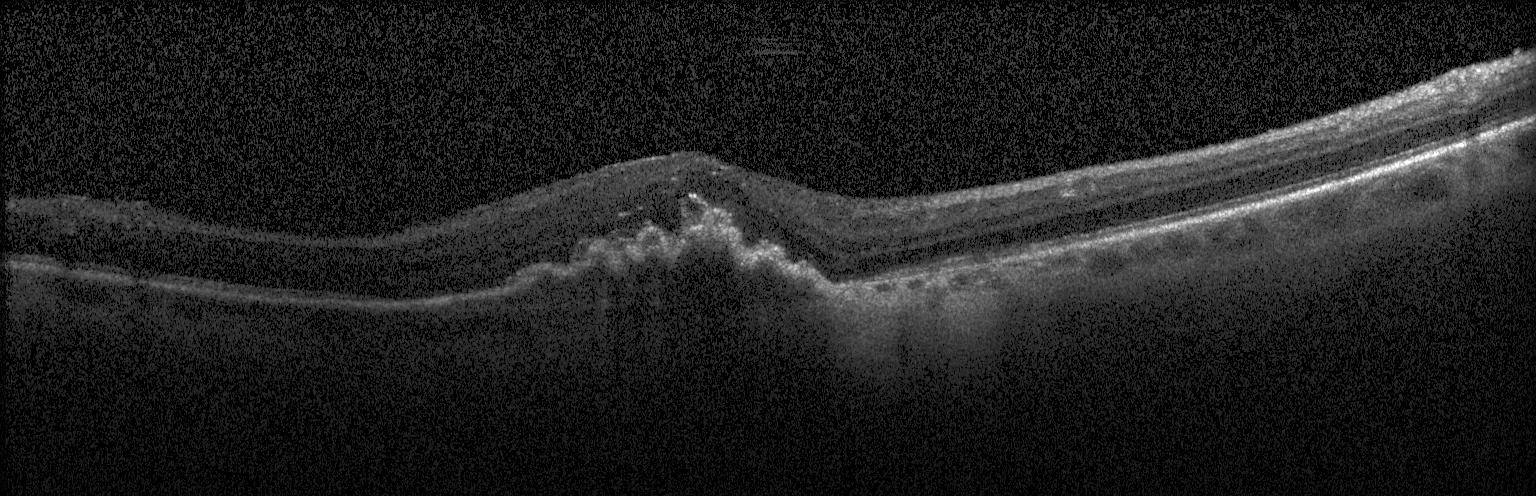 Retinal OCT B-scan, Heidelberg Spectralis OCT system, SD-OCT. Macular OCT: a choroidal neovascular membrane.